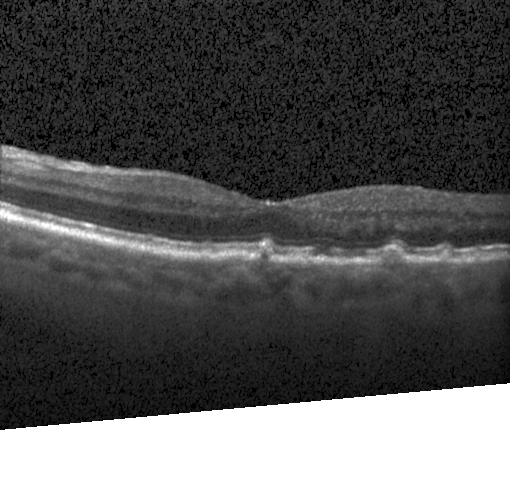 Diagnosis: sub-RPE drusenoid deposits.